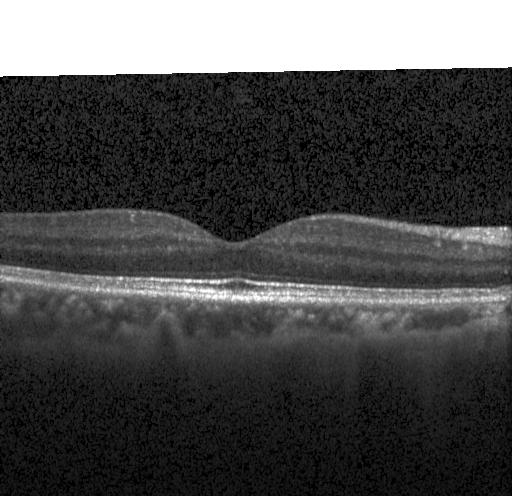 OCT line scan; macular scan; spectral-domain optical coherence tomography.
The scan shows neither choroidal neovascularization, diabetic macular edema, nor drusen.